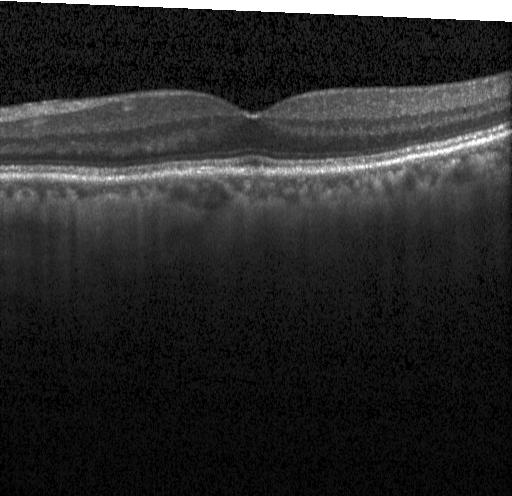 Optical coherence tomography B-scan
Diagnosis: no choroidal neovascularization, no diabetic macular edema, and no drusen.